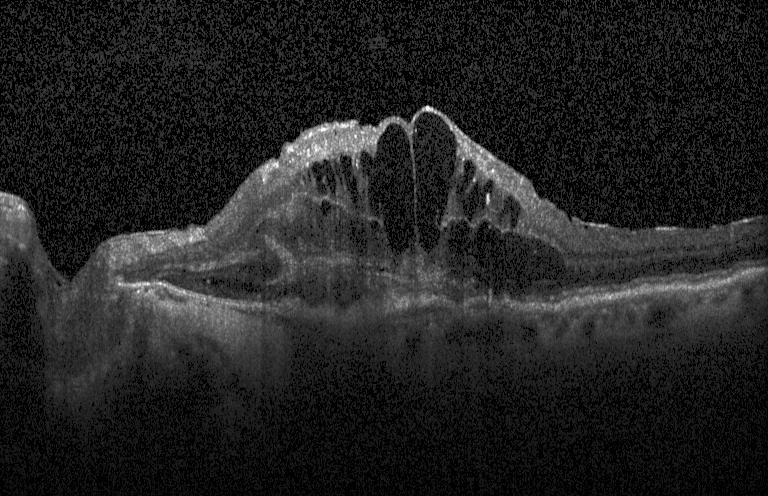 Spectral-domain optical coherence tomography. OCT B-scan. Assessment: choroidal neovascularization.